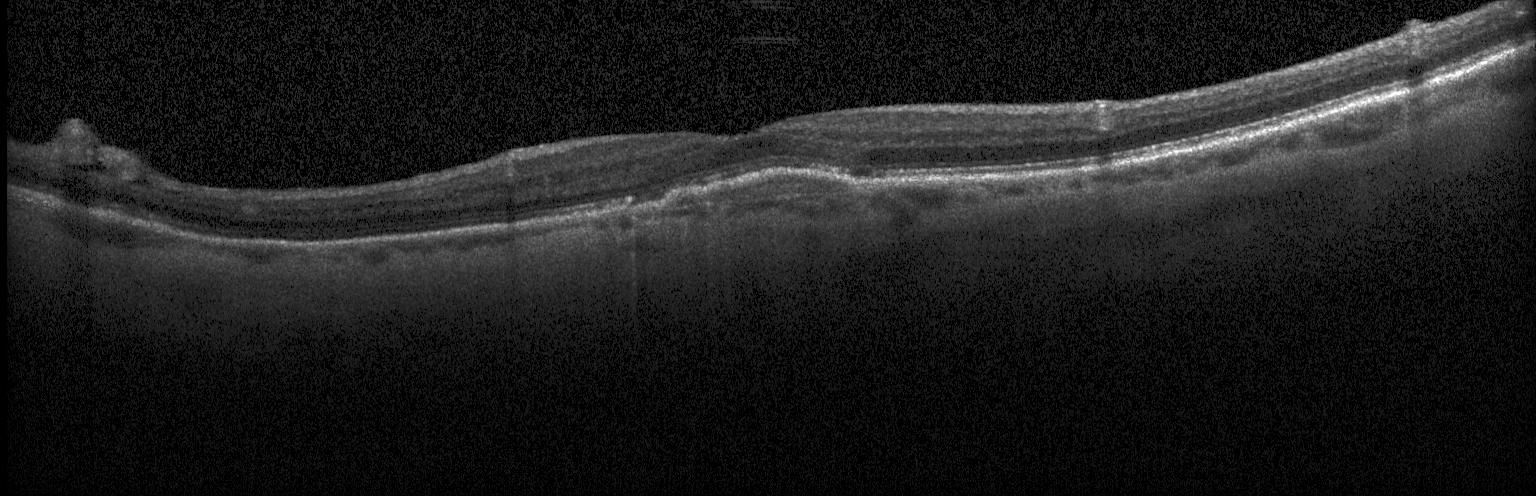
Macular OCT demonstrating choroidal neovascularization.